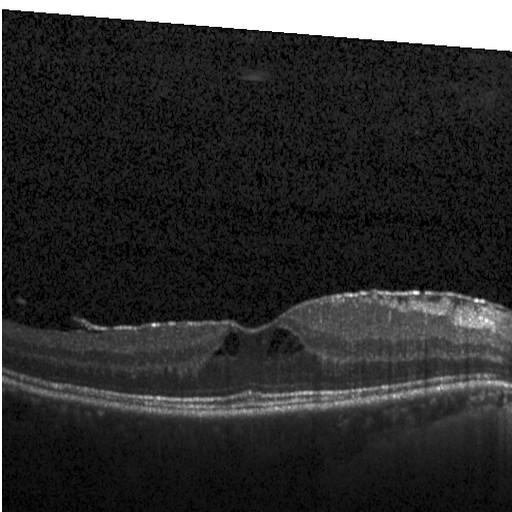
Horizontal scan through the fovea · retinal OCT B-scan · SD-OCT.
The scan shows diabetic macular edema (DME).